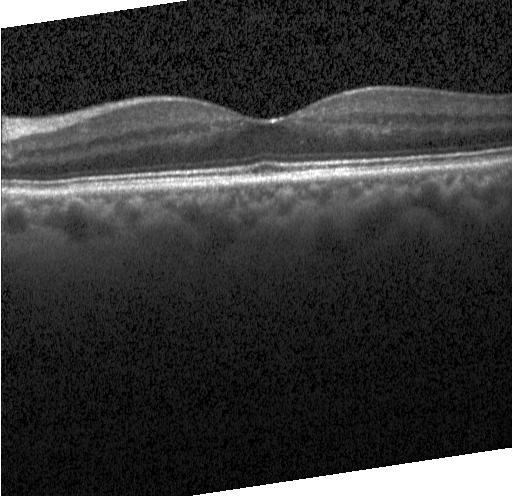

Impression: no choroidal neovascularization, diabetic macular edema, or drusen.